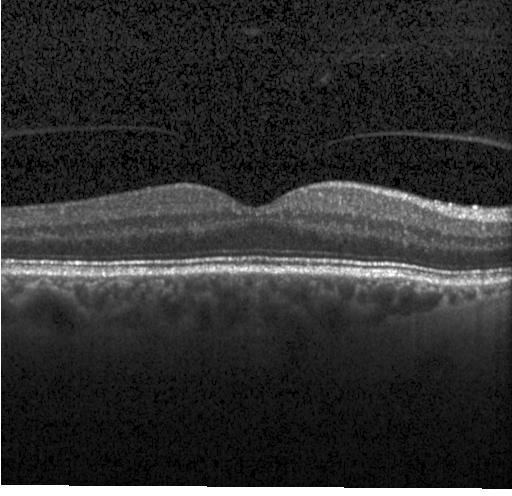
OCT B-scan. Spectral-domain optical coherence tomography. Fovea-centered. Instrument: Heidelberg Spectralis. No CNV, no DME, and no drusen.